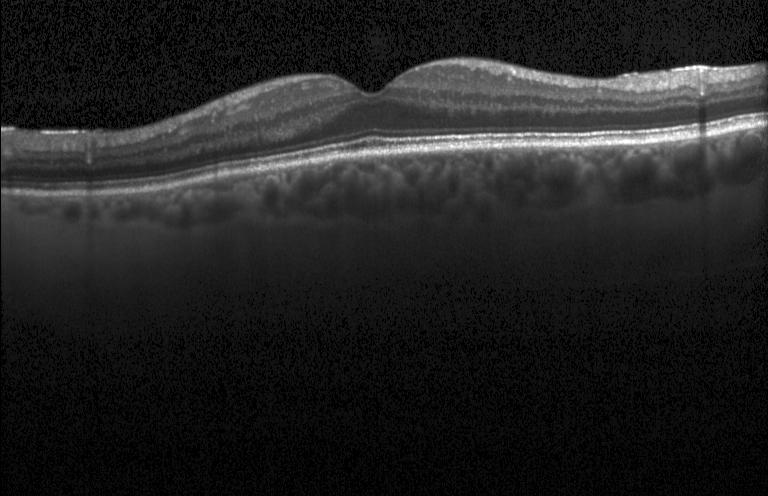

OCT line scan. Macular scan. Impression: neither CNV, DME, nor drusen.